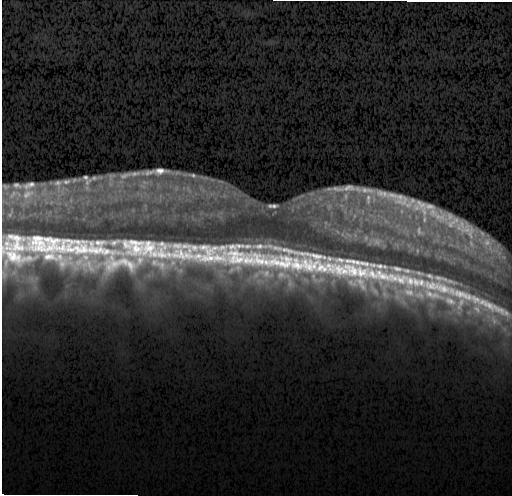
Impression: no CNV, no DME, and no drusen.